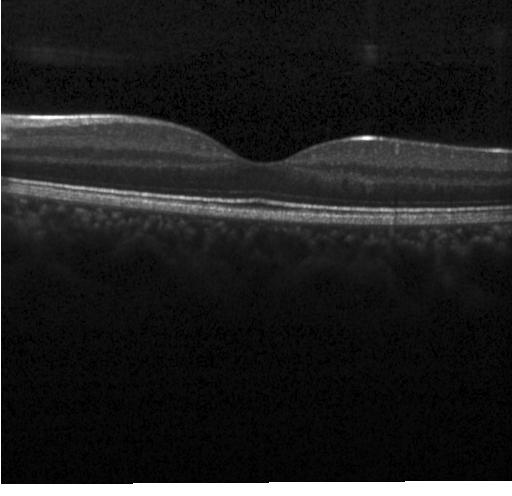 Macular OCT demonstrating no CNV, DME, or drusen.